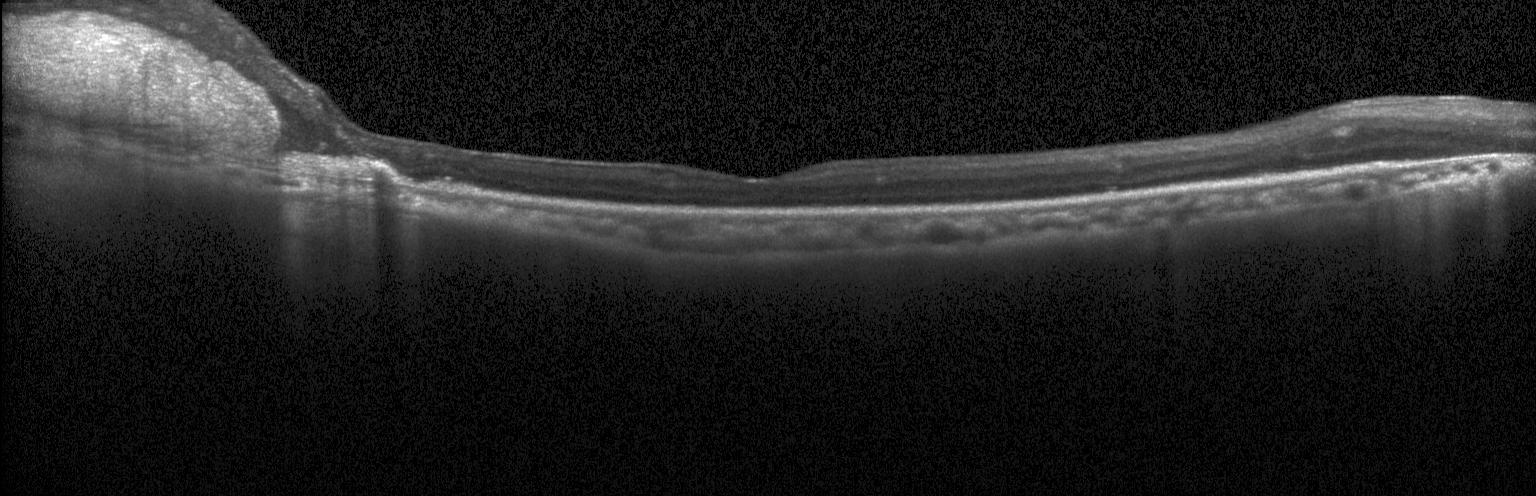 Acquired on a Heidelberg Spectralis. OCT line scan. Impression: a choroidal neovascular membrane.